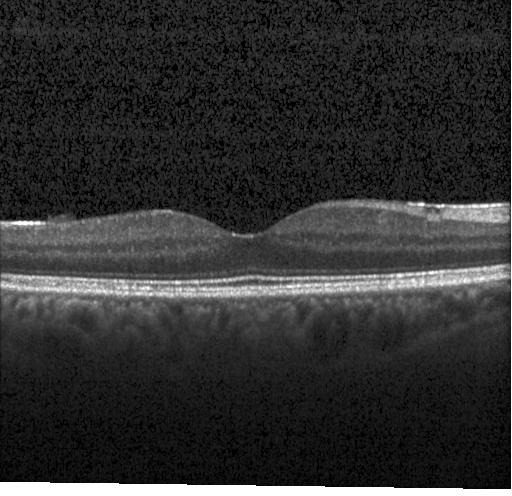
Acquired on a Heidelberg Spectralis, spectral-domain optical coherence tomography, macular scan, retinal OCT cross-section — Macular OCT: no choroidal neovascularization, diabetic macular edema, or drusen.